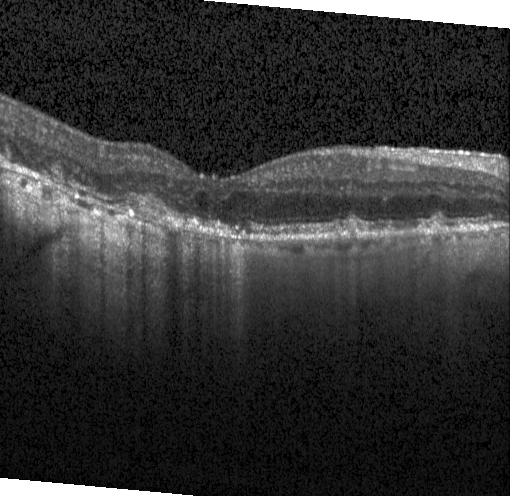

Retinal OCT B-scan. Spectral-domain optical coherence tomography. Instrument: Heidelberg Spectralis. Assessment: choroidal neovascularization (CNV).